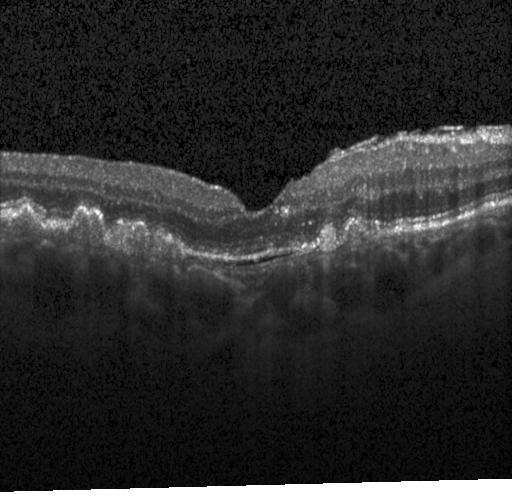 OCT finding: CNV.